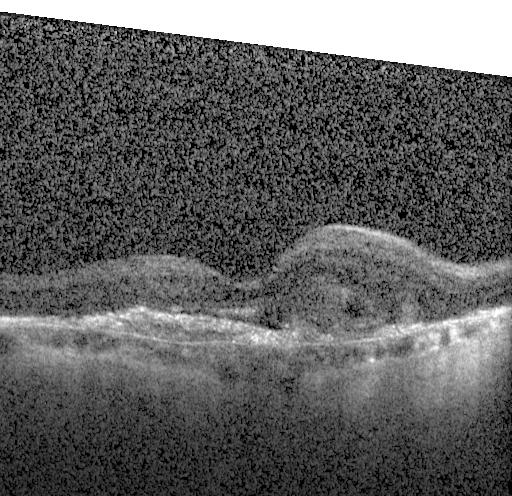
Heidelberg Spectralis OCT system. Optical coherence tomography scan. Spectral-domain optical coherence tomography — This B-scan demonstrates a choroidal neovascular membrane.